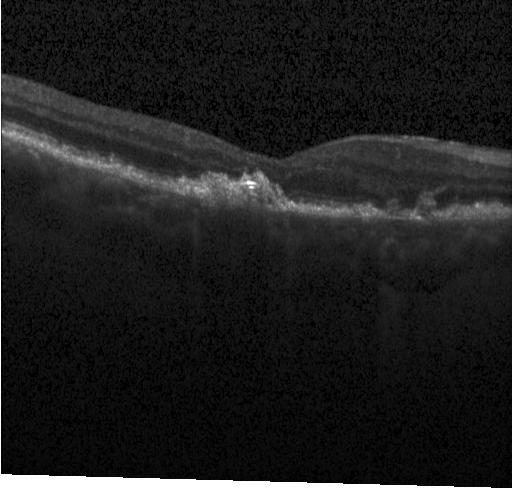
Optical coherence tomography scan; Heidelberg Spectralis
OCT finding: CNV.